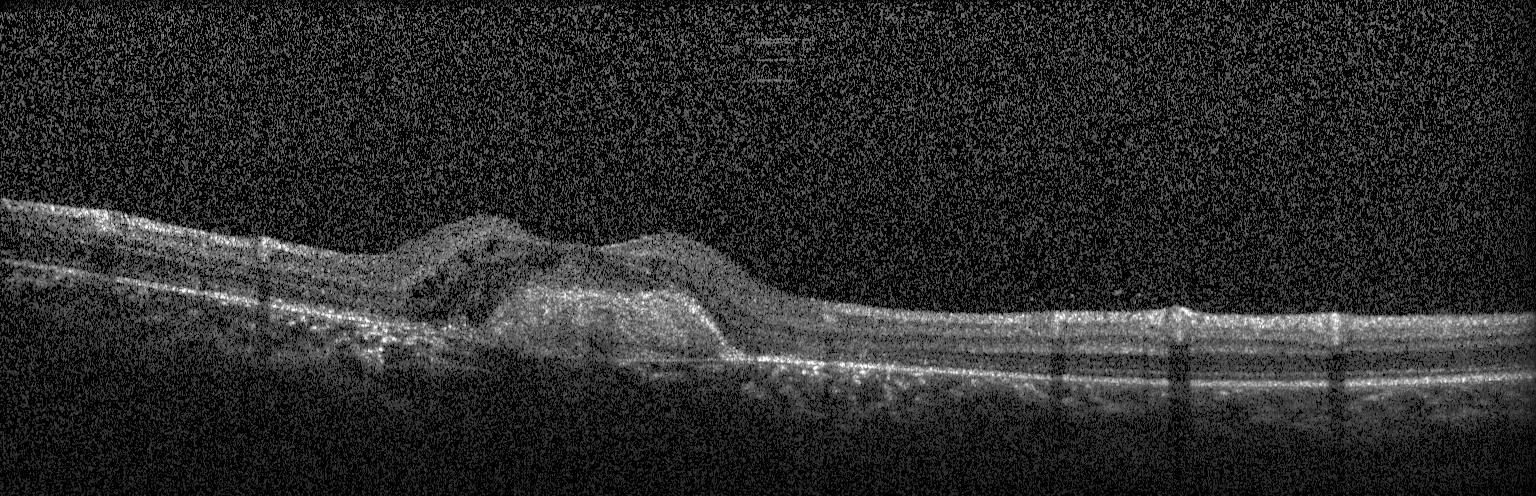 Through the macula · Heidelberg Spectralis OCT system · OCT line scan
Impression: choroidal neovascularization (CNV).